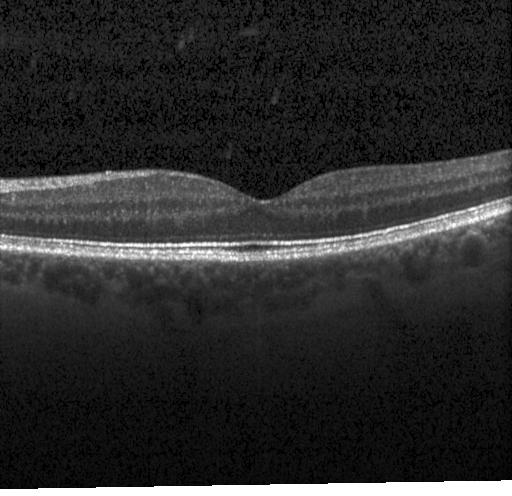 Optical coherence tomography B-scan, SD-OCT, horizontal scan through the fovea, instrument: Heidelberg Spectralis. Impression: no evidence of choroidal neovascularization, diabetic macular edema, or drusen.